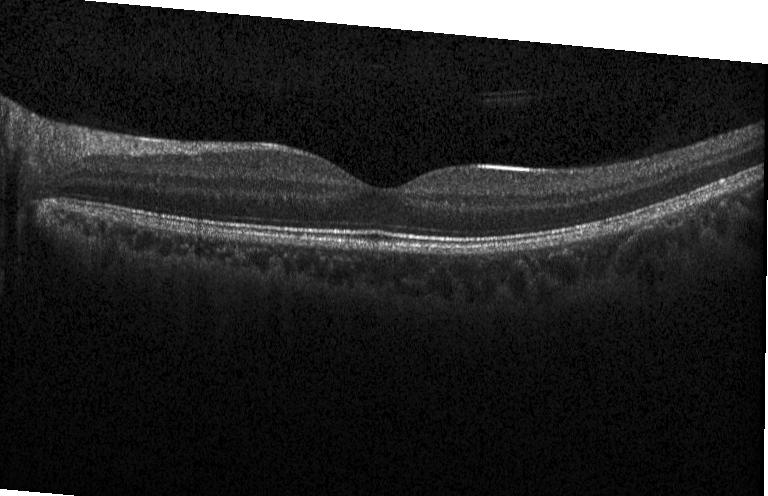

OCT line scan — This B-scan demonstrates neither CNV, DME, nor drusen.